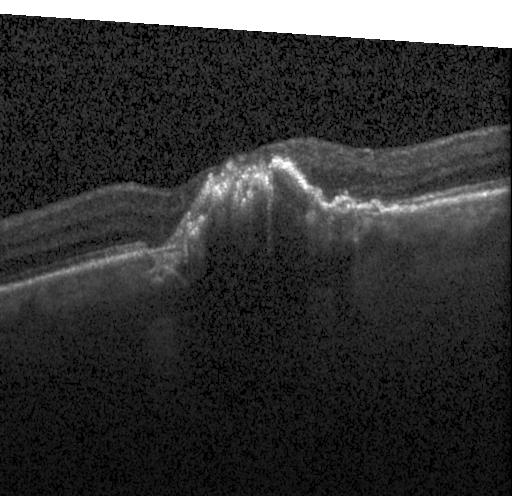 This B-scan demonstrates choroidal neovascularization (CNV).